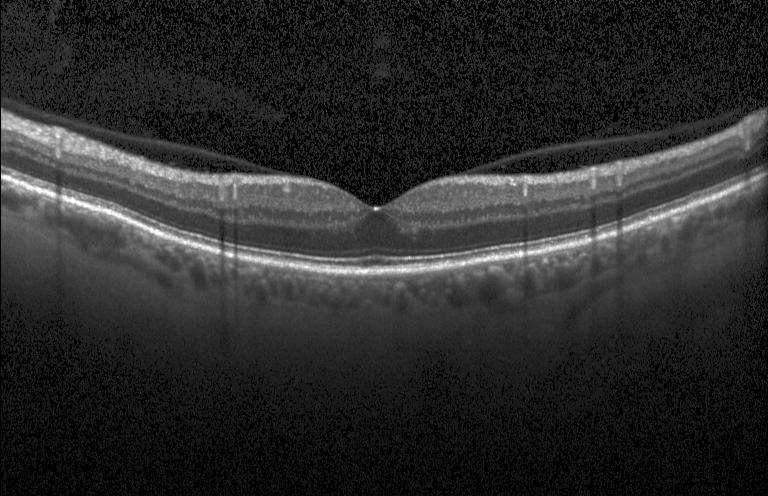 Retinal OCT B-scan, acquired on a Heidelberg Spectralis — Macular OCT: no choroidal neovascularization, diabetic macular edema, or drusen.